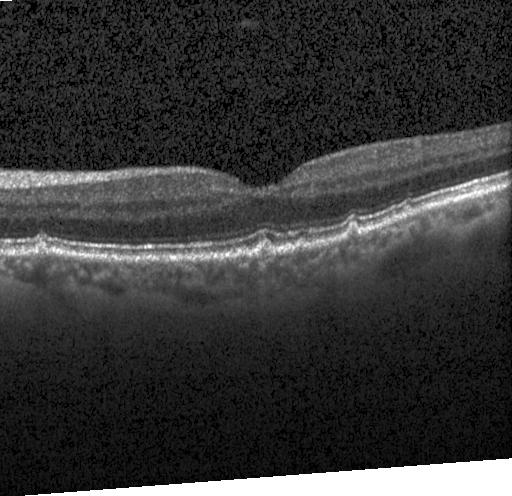
Horizontal scan through the fovea · spectral-domain OCT · Heidelberg Spectralis · optical coherence tomography scan — Macular OCT: multiple drusen.